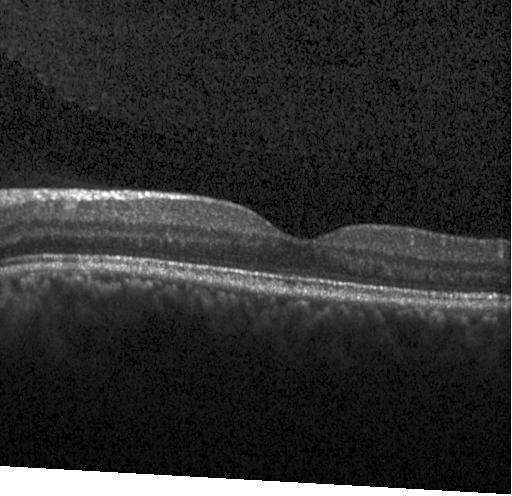

Retinal OCT cross-section showing neither choroidal neovascularization, diabetic macular edema, nor drusen.